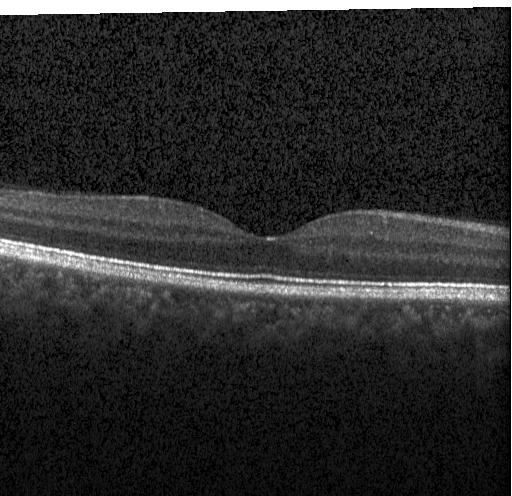
Heidelberg Spectralis · SD-OCT · optical coherence tomography B-scan. Finding: no choroidal neovascularization, no diabetic macular edema, and no drusen.